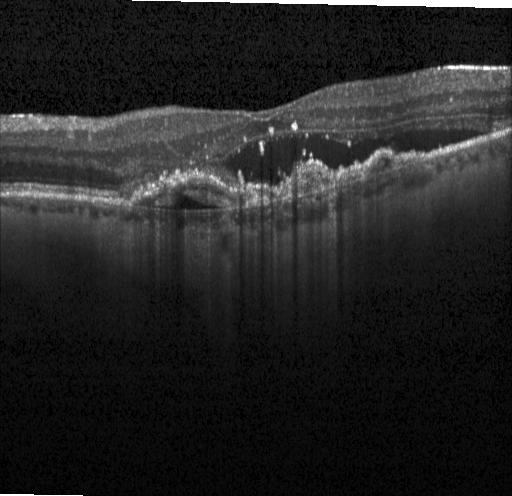
Finding: choroidal neovascularization.